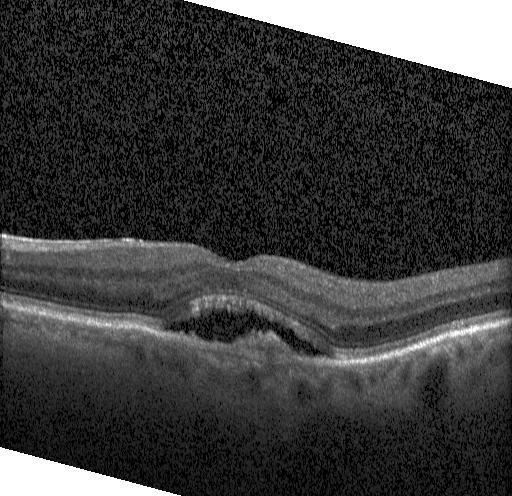
Impression: a choroidal neovascular membrane.